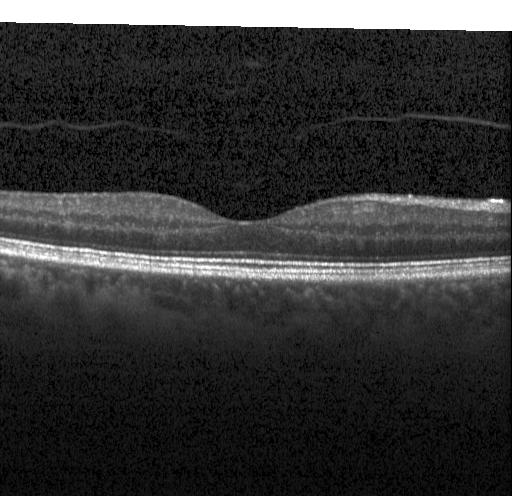
Diagnosis: no CNV, no DME, and no drusen.